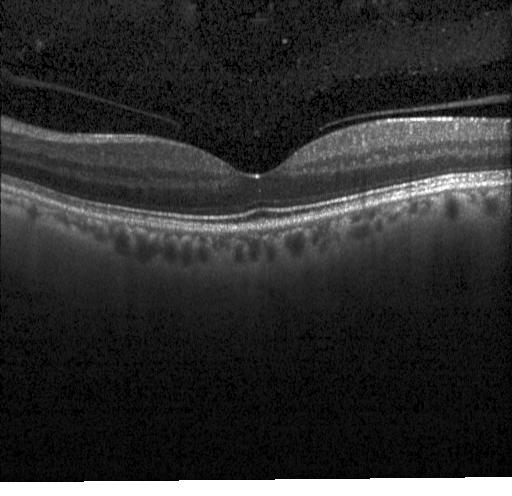 OCT B-scan. SD-OCT — Impression: no evidence of choroidal neovascularization, diabetic macular edema, or drusen.